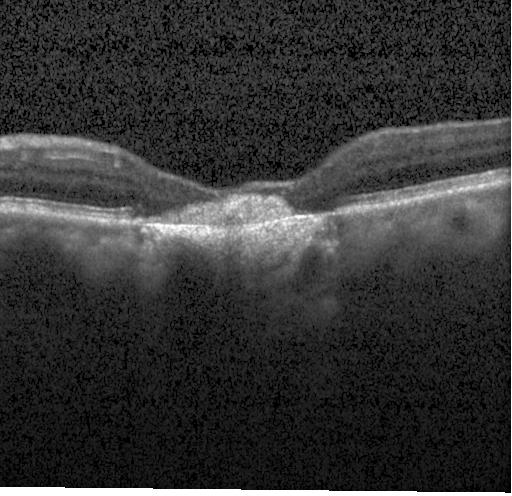
Instrument: Heidelberg Spectralis, spectral-domain optical coherence tomography, retinal OCT B-scan — Diagnosis: a choroidal neovascular membrane.